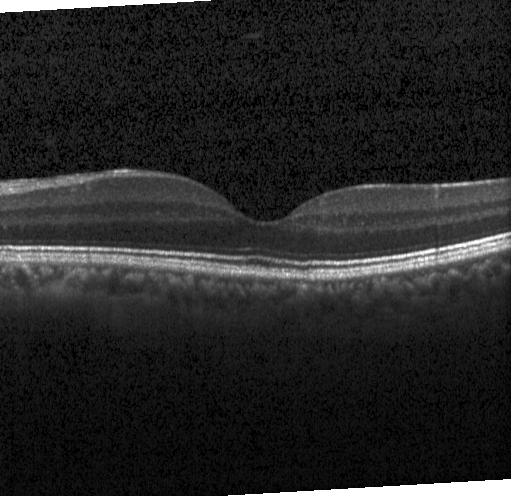
Finding: neither choroidal neovascularization, diabetic macular edema, nor drusen.